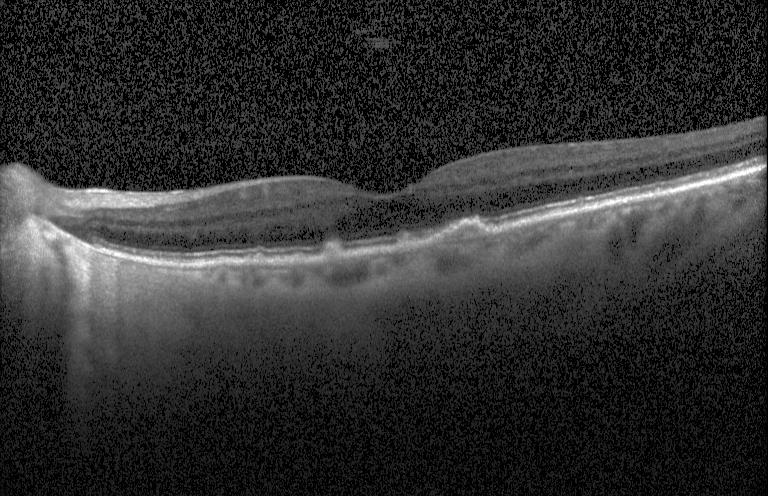
Spectral-domain optical coherence tomography, Heidelberg Spectralis OCT system, OCT B-scan.
OCT finding: choroidal neovascularization.